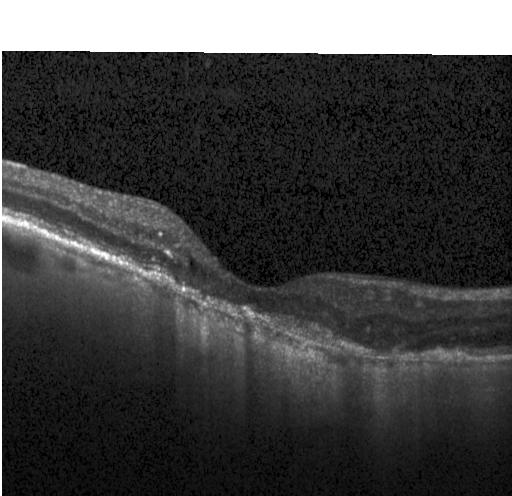 Spectral-domain OCT; retinal OCT cross-section
This B-scan demonstrates CNV.